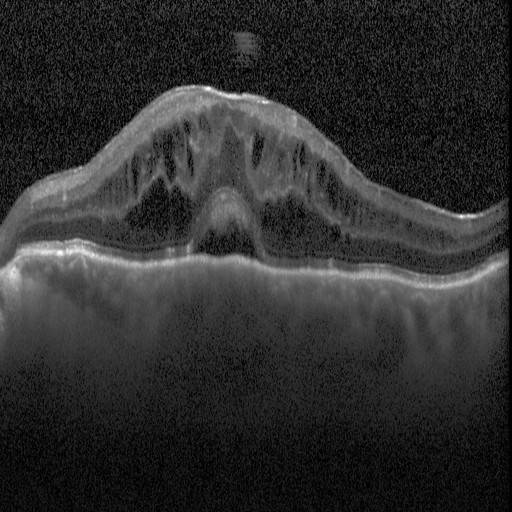
Optical coherence tomography scan · spectral-domain optical coherence tomography — Impression: DME.